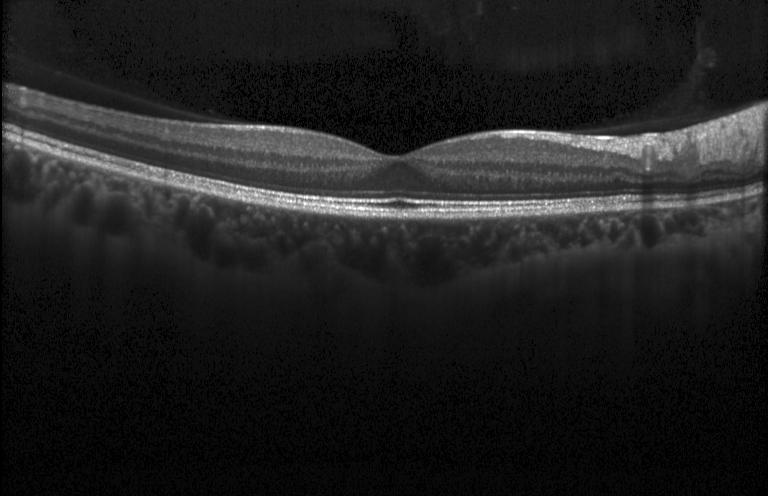
Retinal OCT cross-section showing no evidence of CNV, DME, or drusen.